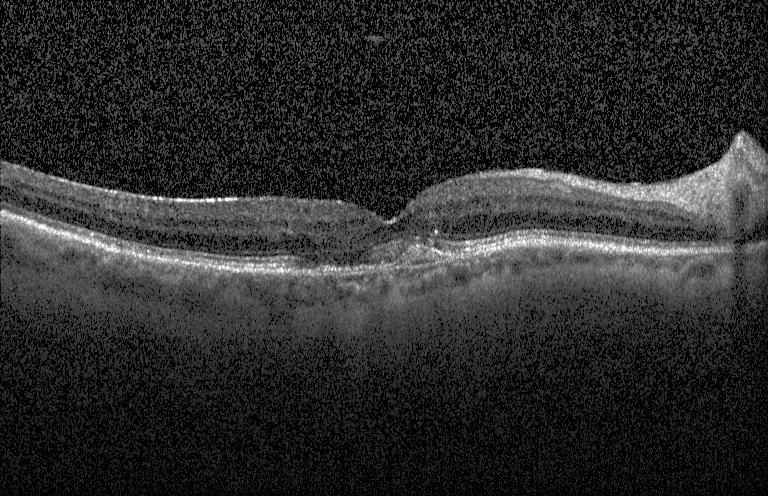
Optical coherence tomography B-scan. Spectral-domain OCT. Horizontal scan through the fovea. Instrument: Heidelberg Spectralis
Finding: a choroidal neovascular membrane.